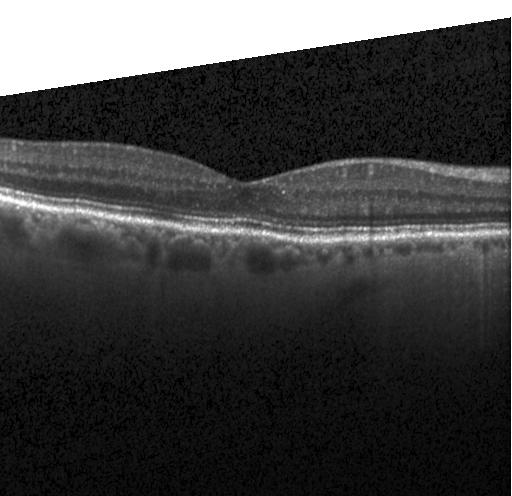

Macular OCT: no evidence of CNV, DME, or drusen.